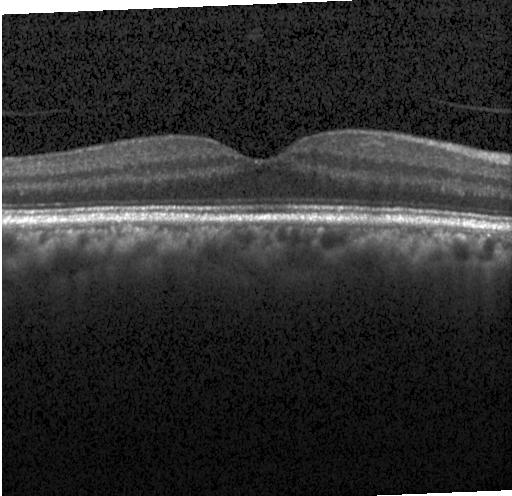 Retinal OCT cross-section. The scan shows no choroidal neovascularization, no diabetic macular edema, and no drusen.